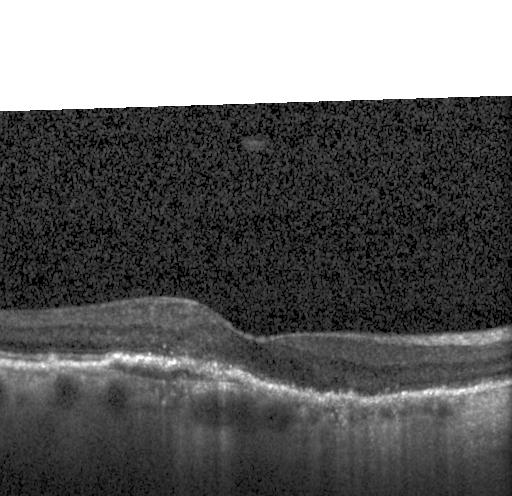

Impression: a choroidal neovascular membrane.